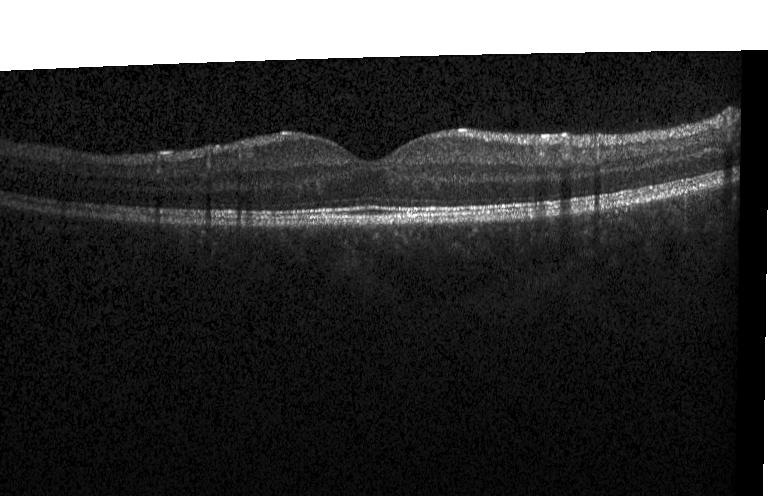

OCT line scan · spectral-domain optical coherence tomography · horizontal scan through the fovea. Impression: no choroidal neovascularization, diabetic macular edema, or drusen.